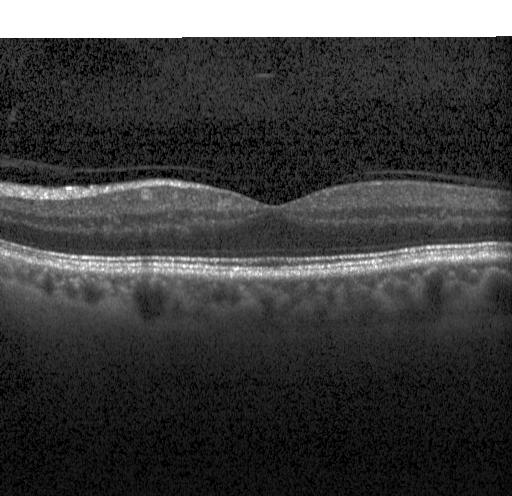
Retinal OCT cross-section. Diagnosis: neither CNV, DME, nor drusen.